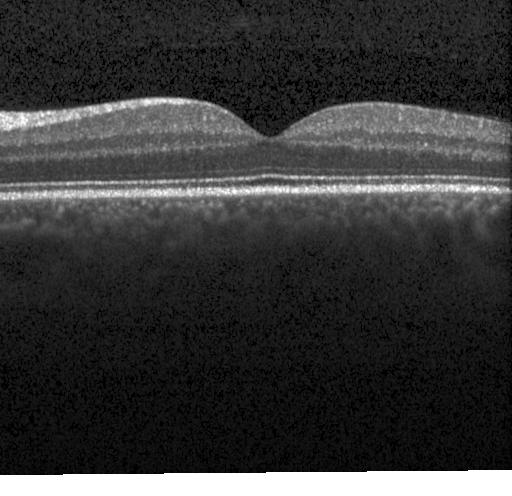

Fovea-centered · SD-OCT · Heidelberg Spectralis · retinal OCT cross-section — Dx: neither CNV, DME, nor drusen.